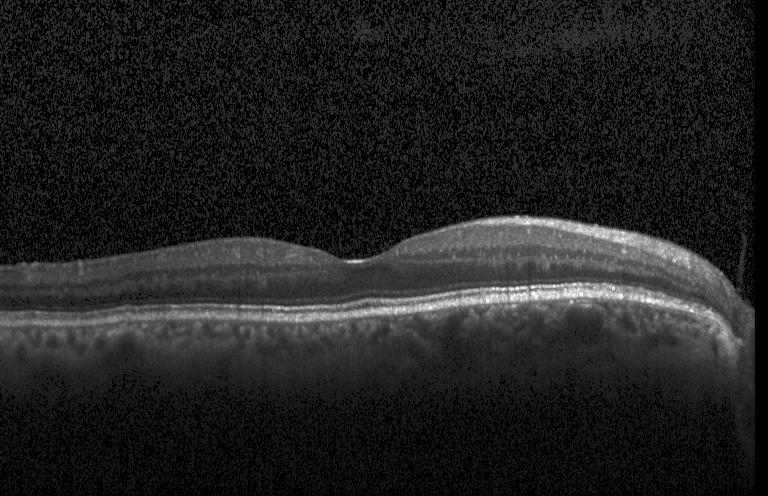
Heidelberg Spectralis · OCT B-scan · SD-OCT
Finding: no choroidal neovascularization, diabetic macular edema, or drusen.